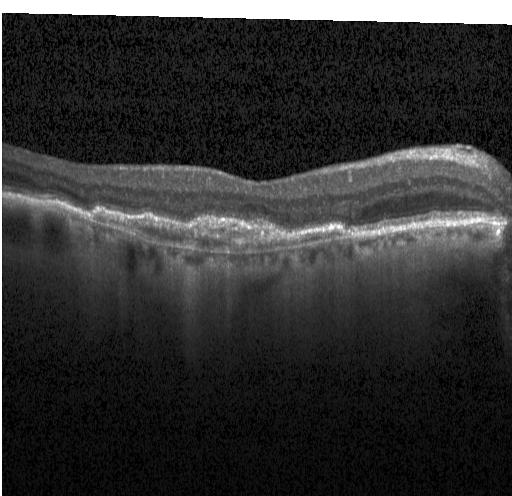

OCT scan showing choroidal neovascularization (CNV).